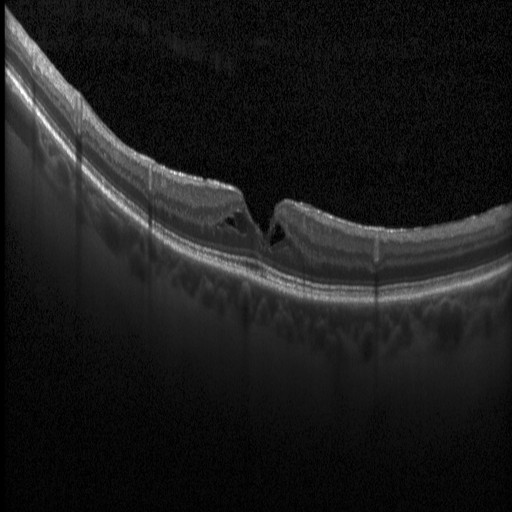
Heidelberg Spectralis · spectral-domain OCT · OCT line scan
OCT finding: diabetic macular edema.